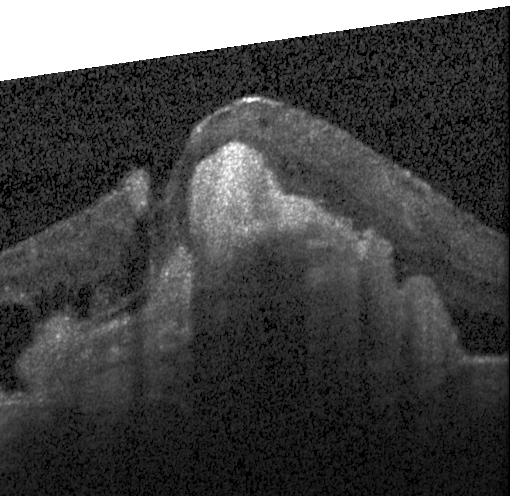
Retinal OCT cross-section showing a choroidal neovascular membrane.